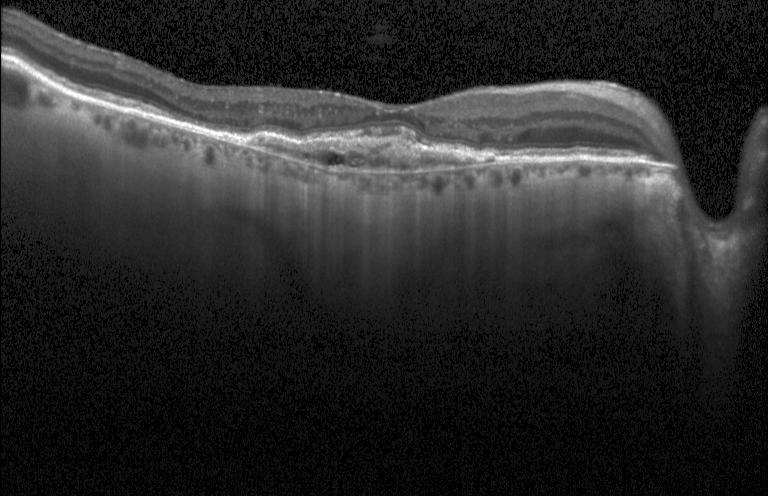

OCT B-scan showing a choroidal neovascular membrane.